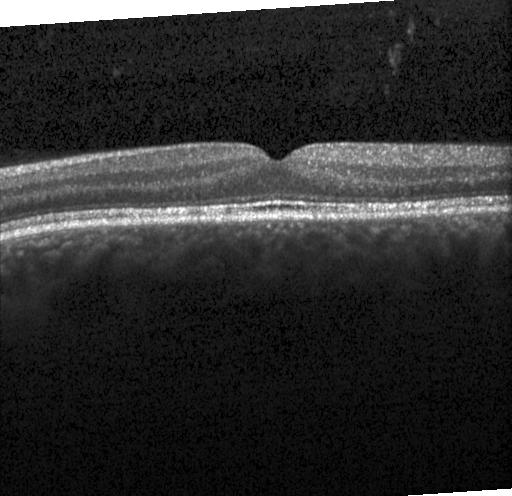

Macular OCT: no evidence of CNV, DME, or drusen.